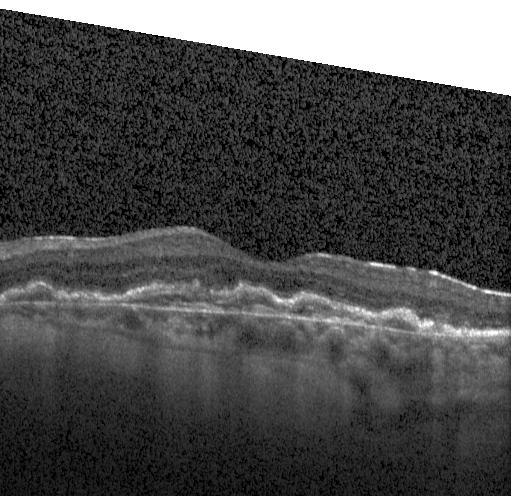
Centered on the fovea. Spectral-domain OCT. OCT line scan. Heidelberg Spectralis — OCT finding: a choroidal neovascular membrane.